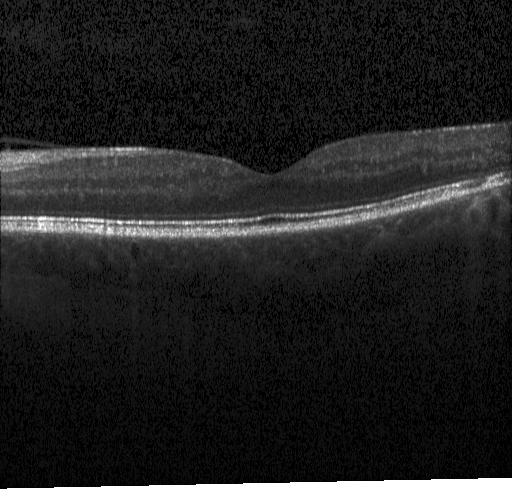

Heidelberg Spectralis. Optical coherence tomography scan. SD-OCT. Centered on the fovea
Impression: neither choroidal neovascularization, diabetic macular edema, nor drusen.